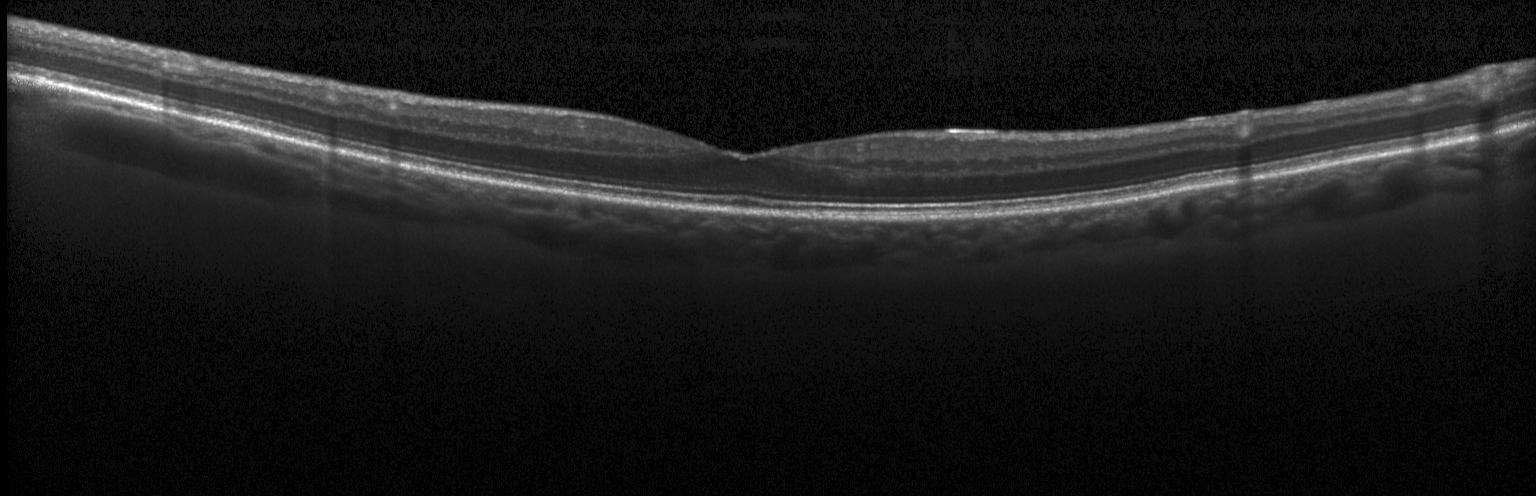
Acquired on a Heidelberg Spectralis; spectral-domain OCT; optical coherence tomography scan
Finding: neither choroidal neovascularization, diabetic macular edema, nor drusen.